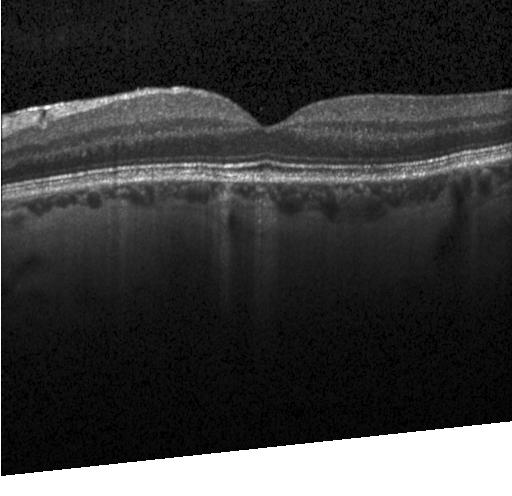

Heidelberg Spectralis OCT system · spectral-domain OCT · macular scan · optical coherence tomography B-scan — Finding: no CNV, no DME, and no drusen.